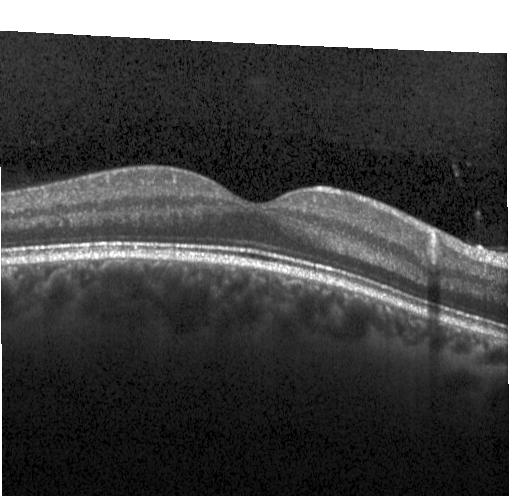
Impression: no choroidal neovascularization, no diabetic macular edema, and no drusen.